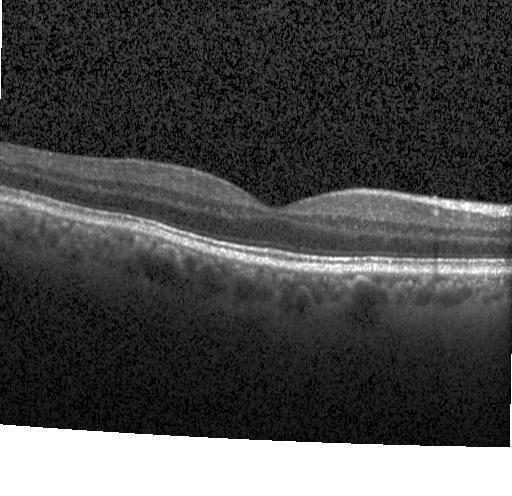
Spectral-domain OCT B-scan: no choroidal neovascularization, no diabetic macular edema, and no drusen.